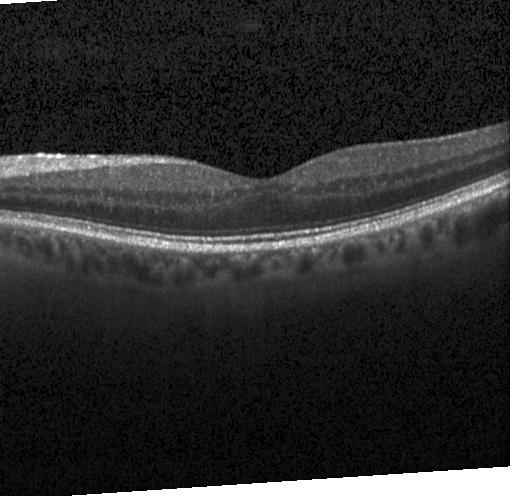

OCT finding: no evidence of choroidal neovascularization, diabetic macular edema, or drusen.